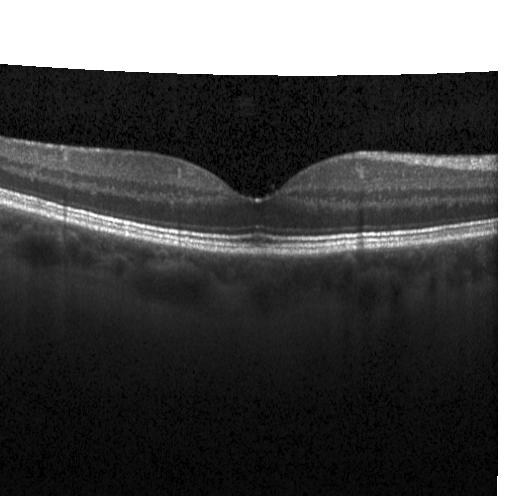 Spectral-domain optical coherence tomography; OCT line scan. The scan shows no evidence of CNV, DME, or drusen.